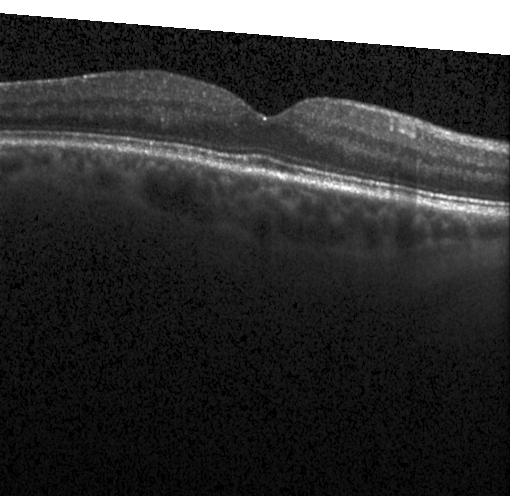

Impression: no choroidal neovascularization, diabetic macular edema, or drusen.